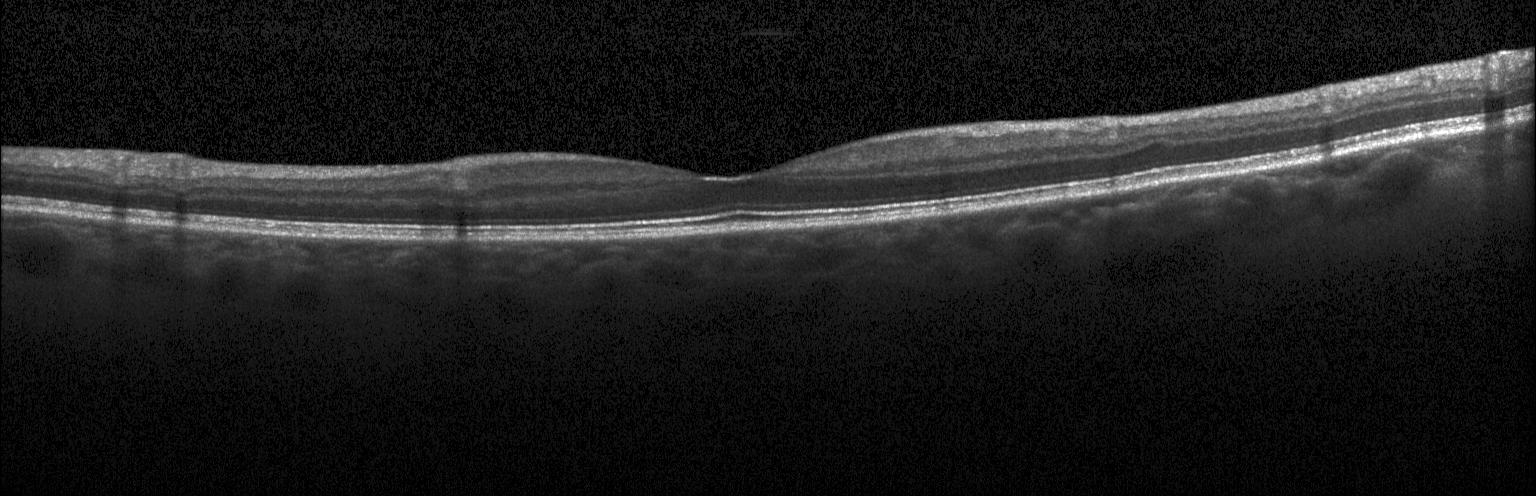
OCT B-scan, instrument: Heidelberg Spectralis
Finding: no CNV, DME, or drusen.